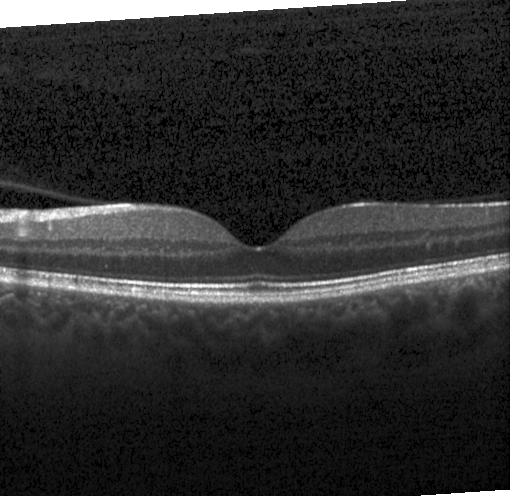 OCT scan showing neither CNV, DME, nor drusen.